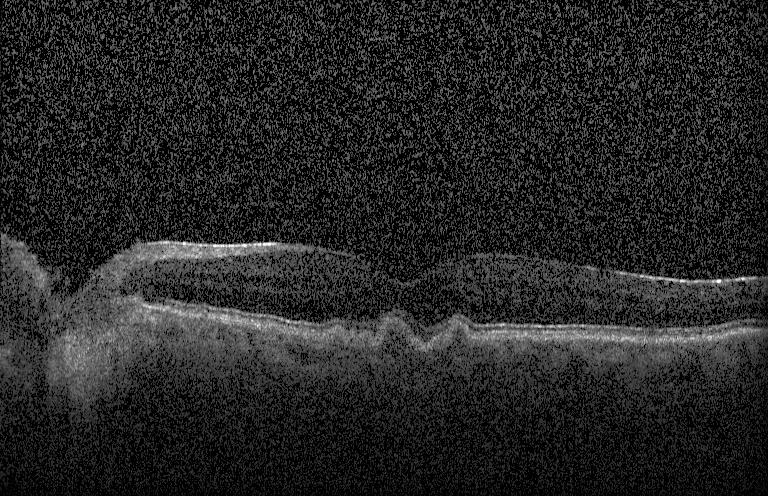

Spectral-domain optical coherence tomography · macular scan · Heidelberg Spectralis · retinal OCT cross-section
Finding: multiple drusen.